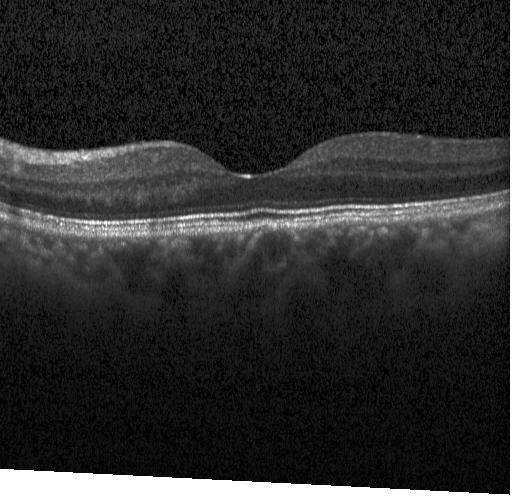
Optical coherence tomography scan. Assessment: no CNV, no DME, and no drusen.